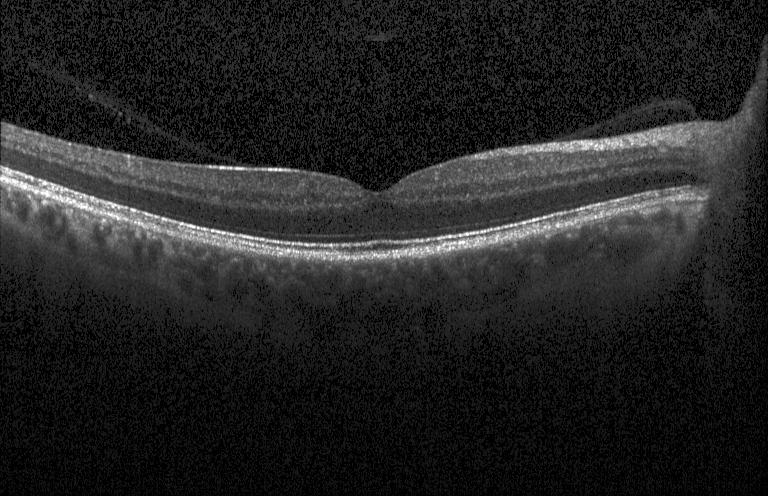
Instrument: Heidelberg Spectralis, optical coherence tomography scan, SD-OCT.
This B-scan demonstrates no evidence of CNV, DME, or drusen.